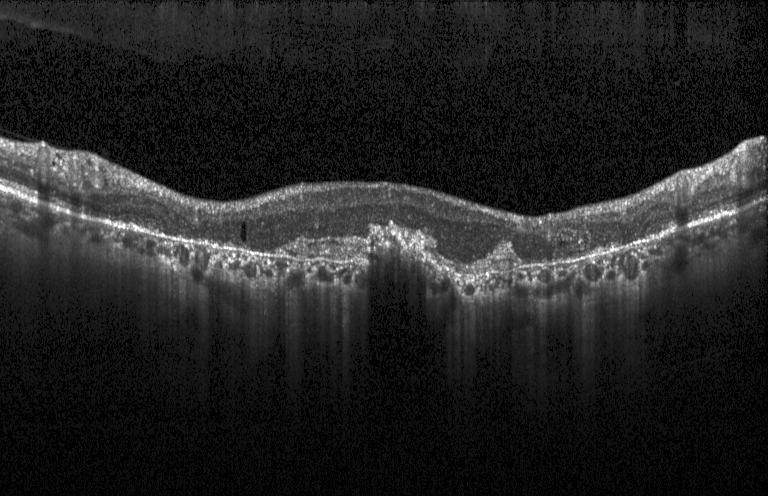
Retinal OCT cross-section
A choroidal neovascular membrane.